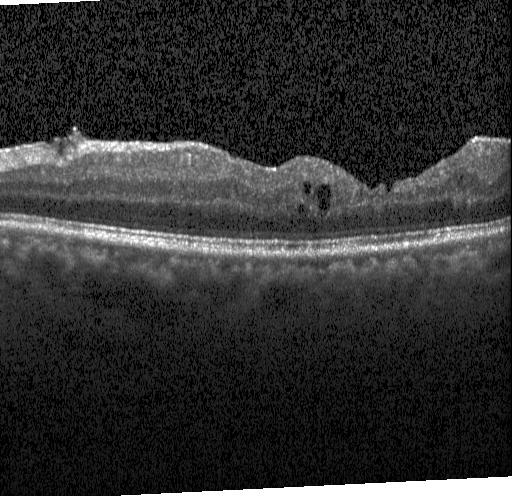 Impression: diabetic macular edema (DME).